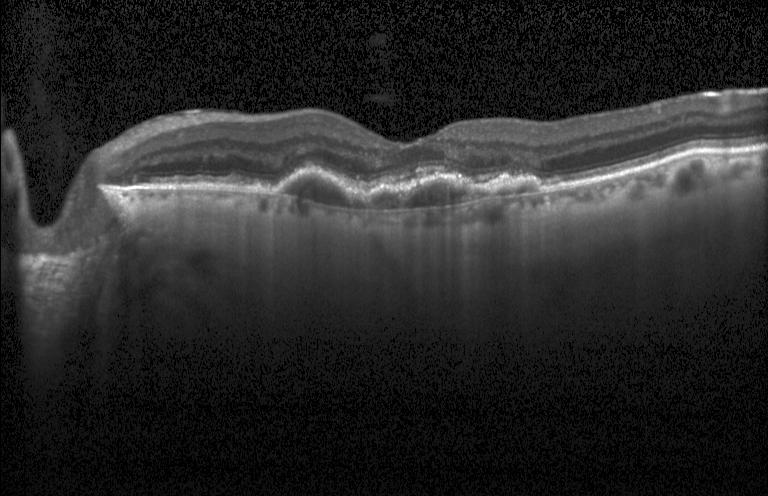 This B-scan demonstrates choroidal neovascularization (CNV).